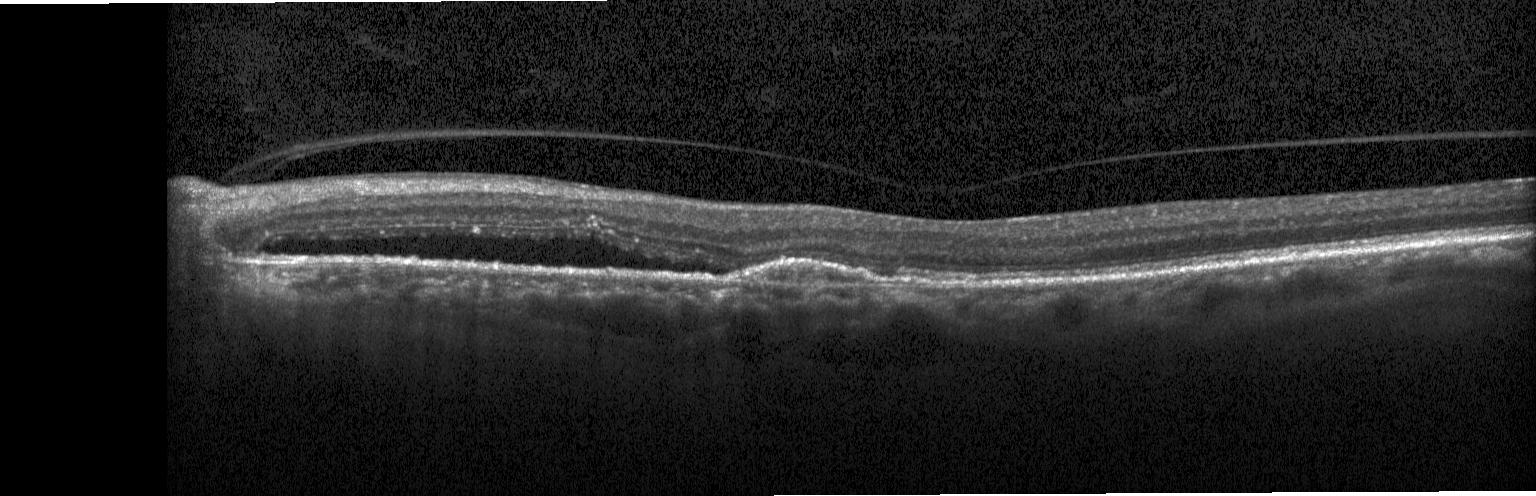 Heidelberg Spectralis OCT system; macular scan; optical coherence tomography scan — Assessment: a choroidal neovascular membrane.